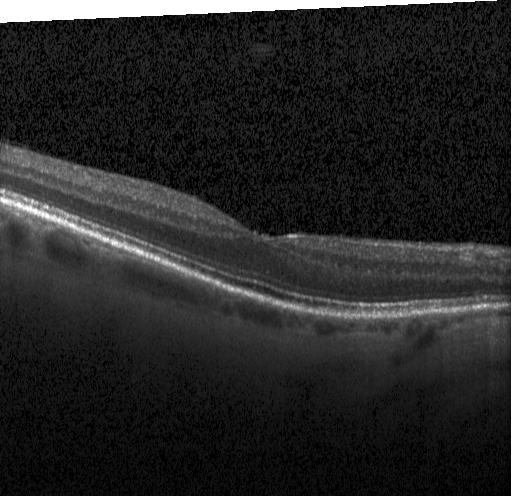
Optical coherence tomography B-scan. Fovea-centered. Spectral-domain OCT. Heidelberg Spectralis. Impression: no CNV, no DME, and no drusen.